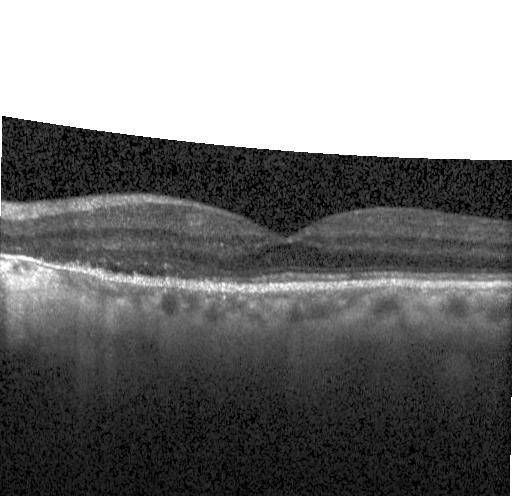
Macular scan, acquired on a Heidelberg Spectralis, optical coherence tomography scan, SD-OCT
This B-scan demonstrates neither choroidal neovascularization, diabetic macular edema, nor drusen.